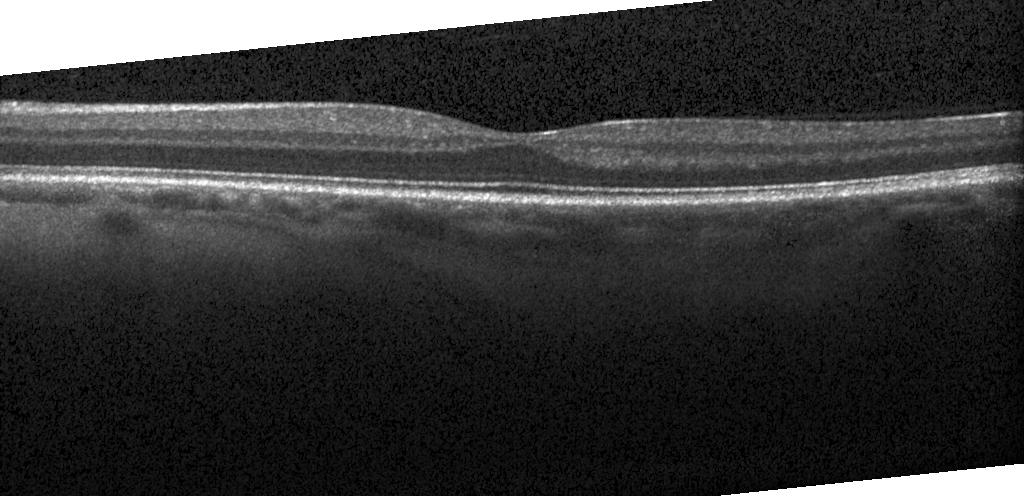 Macular OCT demonstrating no evidence of CNV, DME, or drusen.